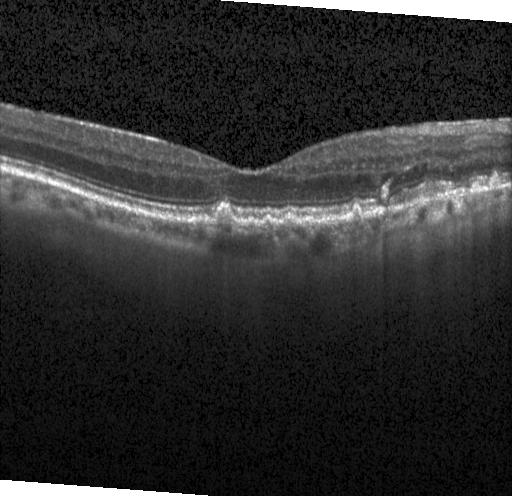
Spectral-domain optical coherence tomography; fovea-centered; OCT B-scan — Sub-RPE drusenoid deposits.